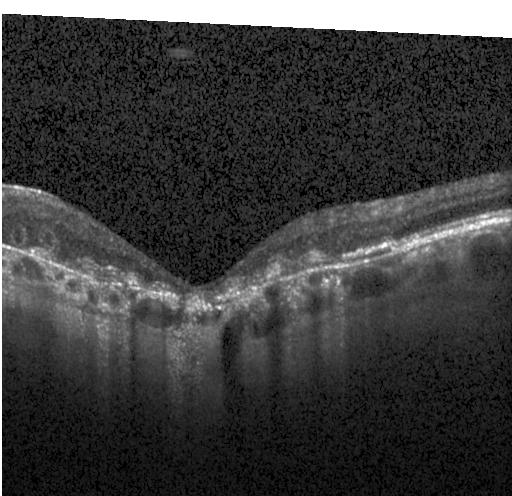
Retinal OCT cross-section showing a choroidal neovascular membrane.